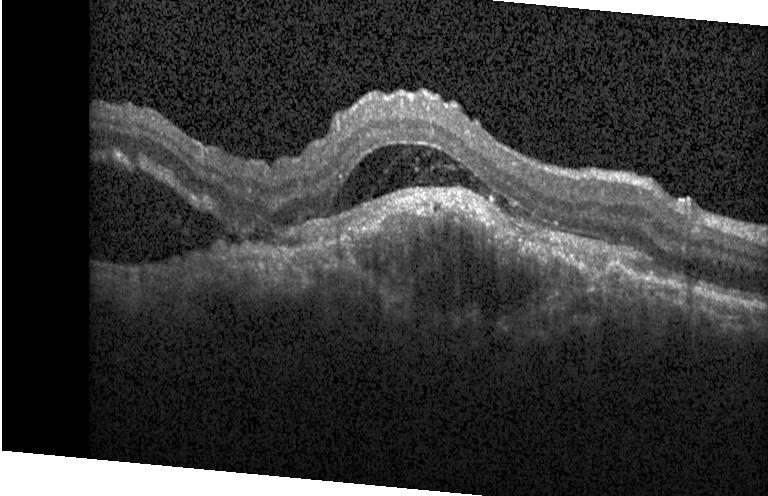

Spectral-domain optical coherence tomography. OCT B-scan. Fovea-centered
This B-scan demonstrates choroidal neovascularization.